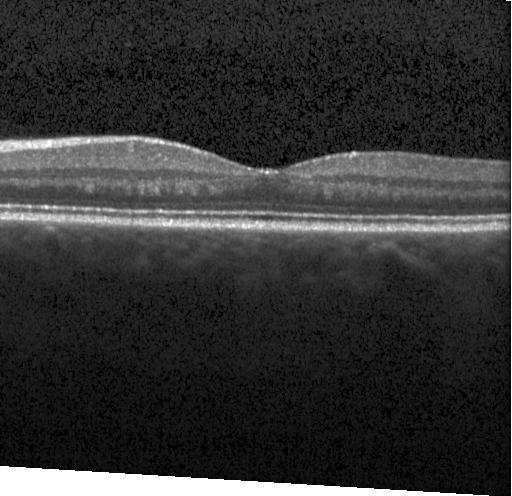

OCT line scan — Finding: neither CNV, DME, nor drusen.